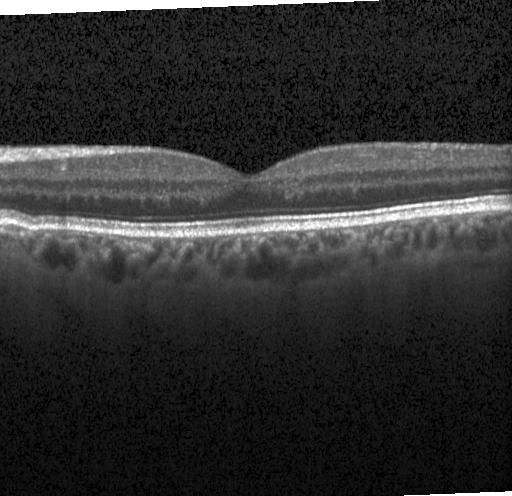 OCT line scan — Dx: no CNV, no DME, and no drusen.